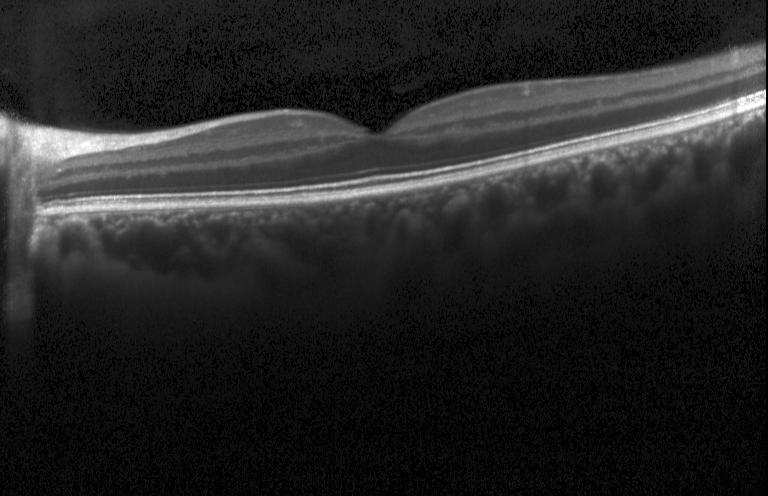
Optical coherence tomography scan; spectral-domain optical coherence tomography; instrument: Heidelberg Spectralis.
Impression: no choroidal neovascularization, no diabetic macular edema, and no drusen.